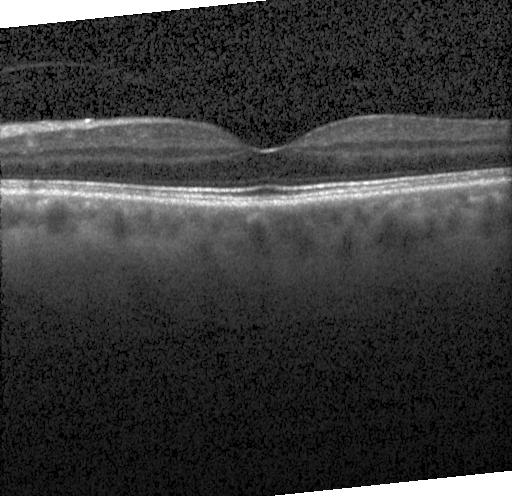

Diagnosis: no evidence of choroidal neovascularization, diabetic macular edema, or drusen.